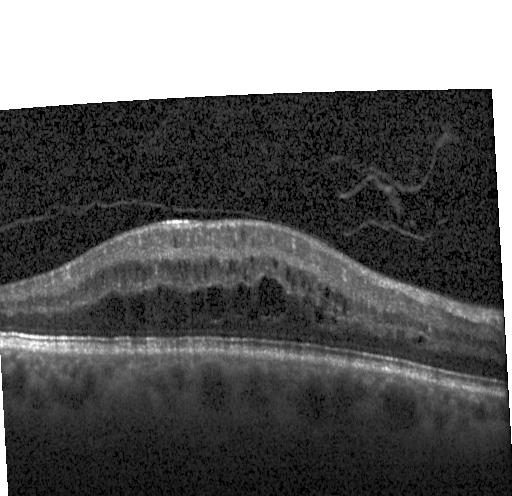

Impression: diabetic macular edema (DME).